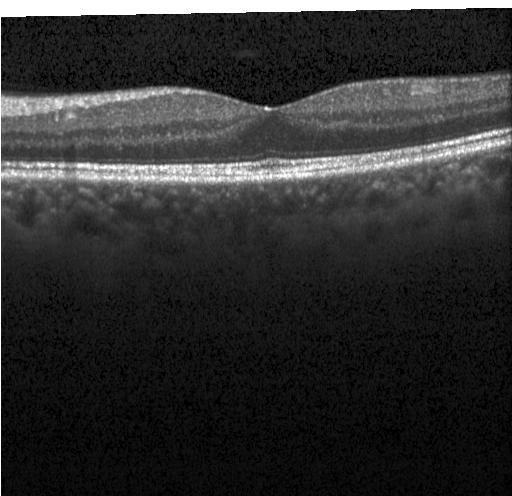 Retinal OCT cross-section; spectral-domain optical coherence tomography
Macular OCT: no evidence of choroidal neovascularization, diabetic macular edema, or drusen.